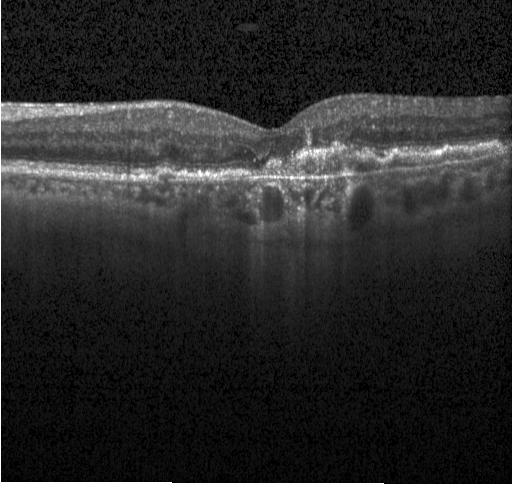 Retinal OCT cross-section · acquired on a Heidelberg Spectralis · through the macula — CNV.